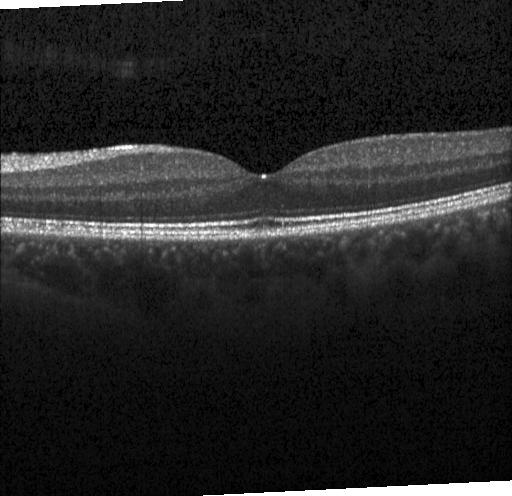
OCT B-scan showing no choroidal neovascularization, diabetic macular edema, or drusen.